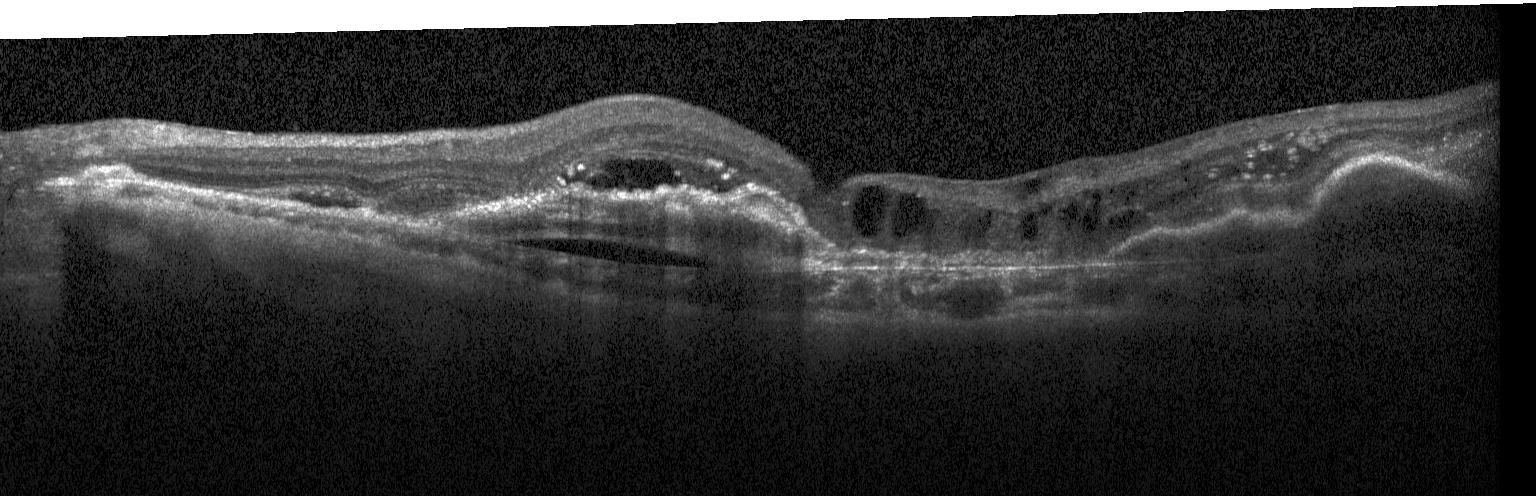
Optical coherence tomography B-scan; through the macula; Heidelberg Spectralis; spectral-domain optical coherence tomography. Choroidal neovascularization.